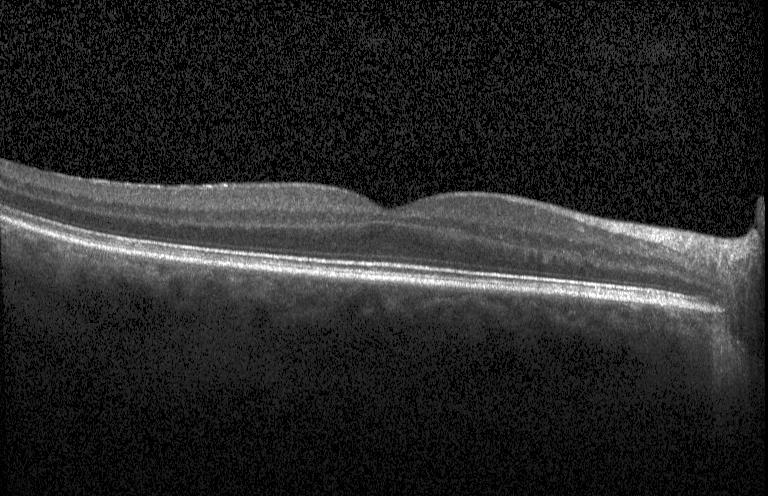

Spectral-domain optical coherence tomography. Through the macula. OCT B-scan. Heidelberg Spectralis OCT system.
Assessment: no choroidal neovascularization, diabetic macular edema, or drusen.